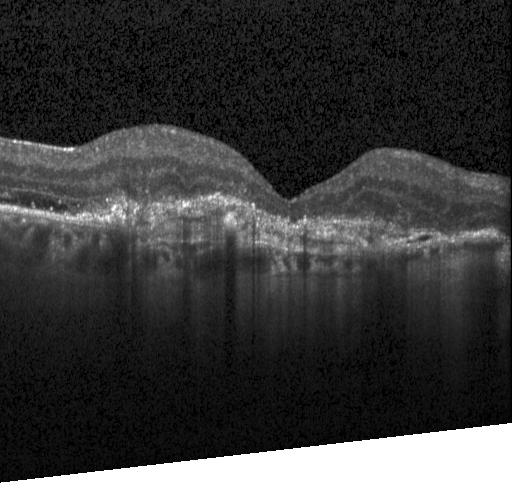 Dx: a choroidal neovascular membrane.